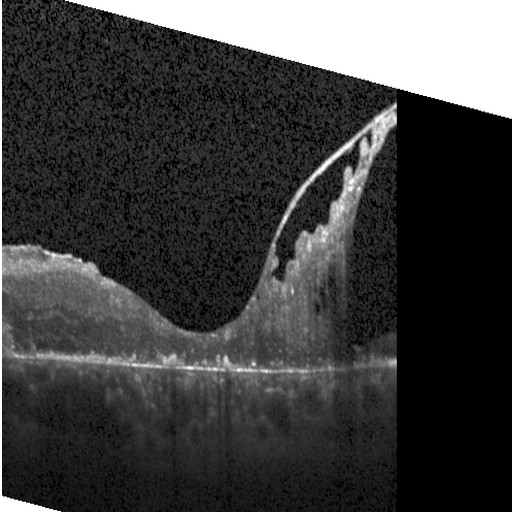 Optical coherence tomography B-scan; spectral-domain optical coherence tomography
Diagnosis: DME.